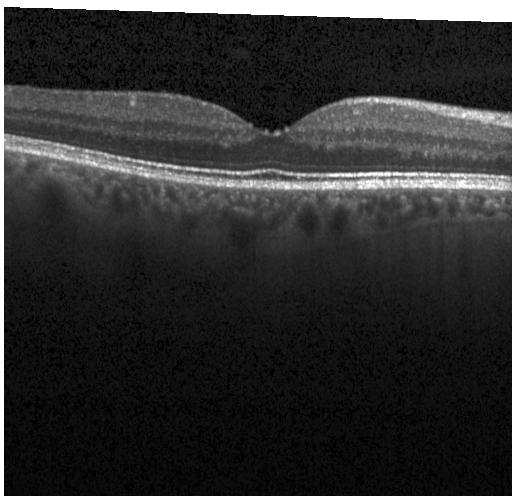

OCT B-scan. Impression: no evidence of choroidal neovascularization, diabetic macular edema, or drusen.